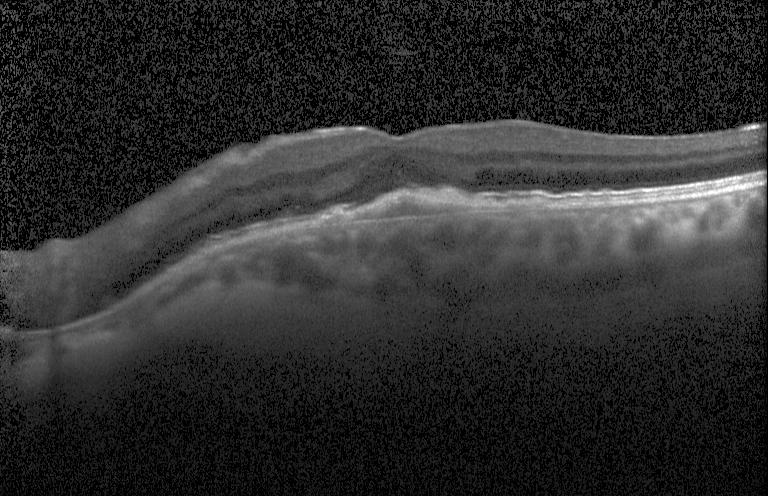

Retinal OCT B-scan, SD-OCT, instrument: Heidelberg Spectralis
Choroidal neovascularization.